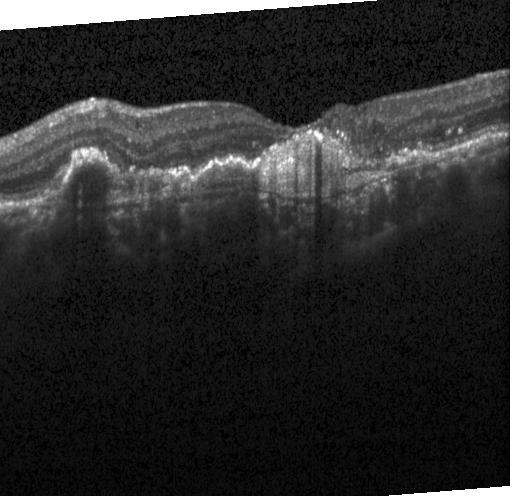 Retinal OCT B-scan — Diagnosis: a choroidal neovascular membrane.